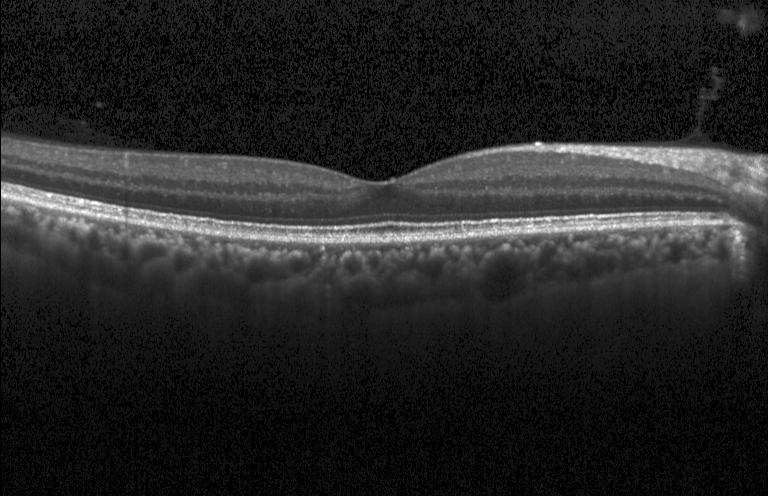 OCT scan showing no choroidal neovascularization, diabetic macular edema, or drusen.